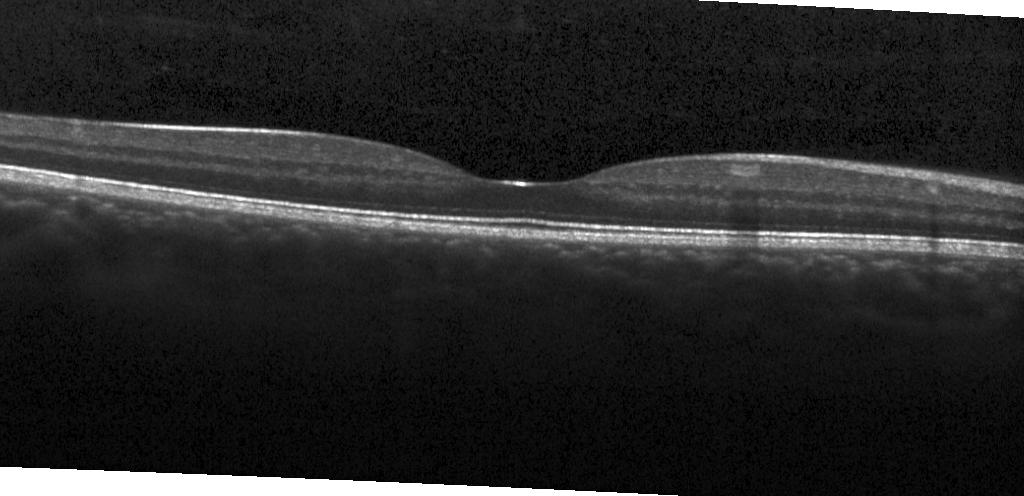 Acquired on a Heidelberg Spectralis; retinal OCT cross-section.
Assessment: no evidence of choroidal neovascularization, diabetic macular edema, or drusen.